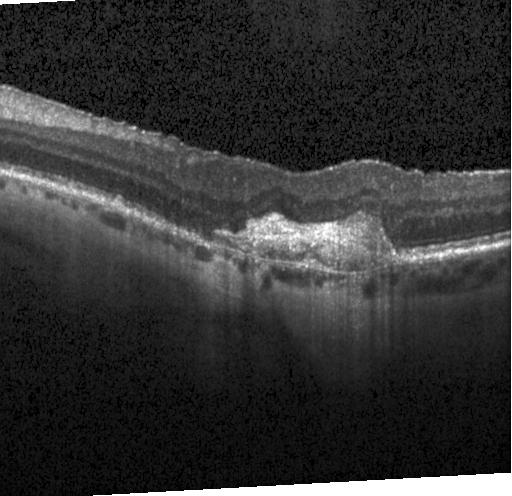

Impression: a choroidal neovascular membrane.